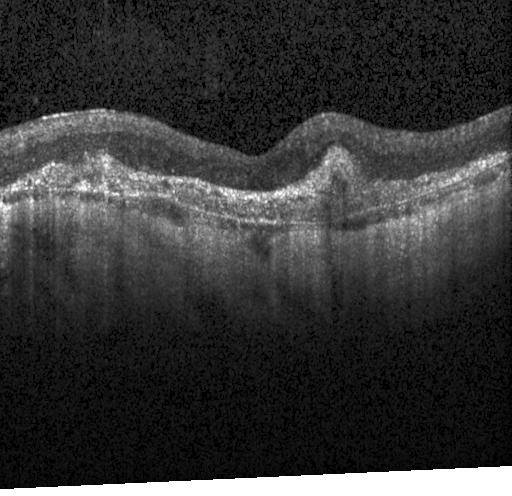
The scan shows CNV.